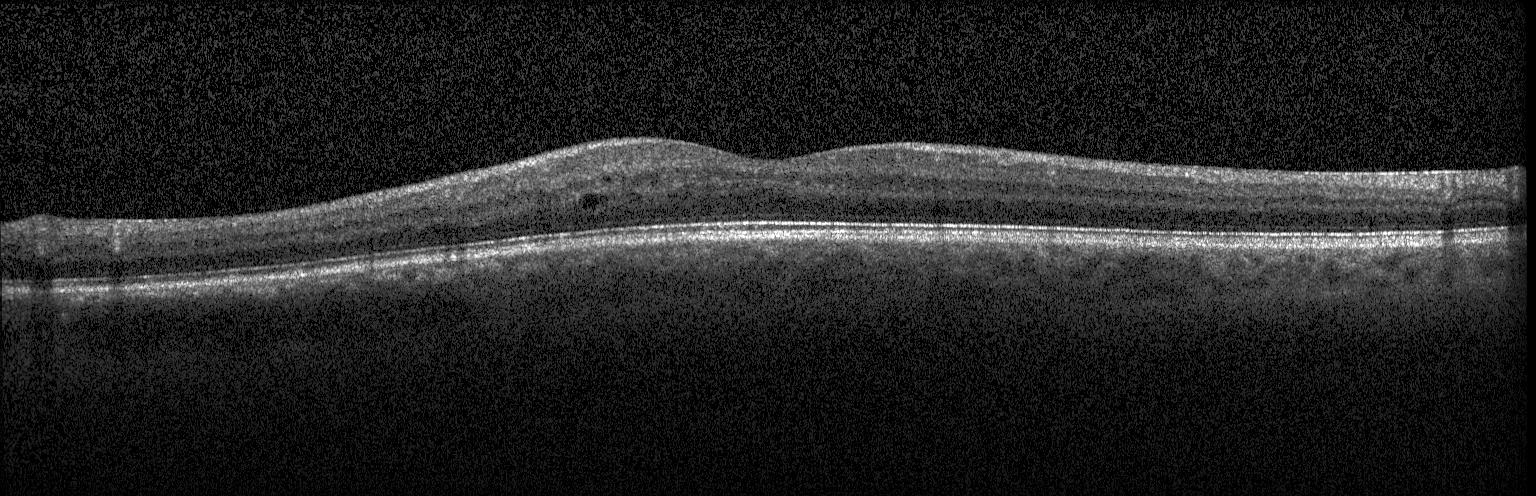
Instrument: Heidelberg Spectralis, spectral-domain optical coherence tomography, horizontal scan through the fovea, retinal OCT B-scan
OCT finding: diabetic macular edema.